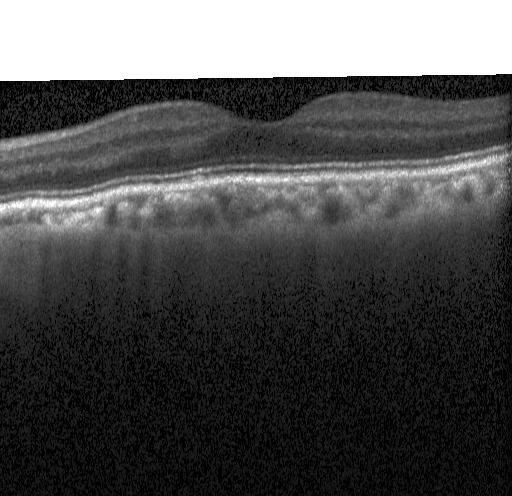
OCT scan showing no CNV, no DME, and no drusen.